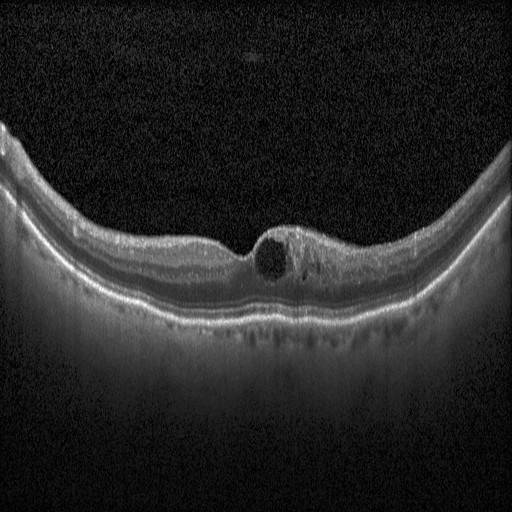
Optical coherence tomography B-scan · spectral-domain optical coherence tomography.
Finding: DME.